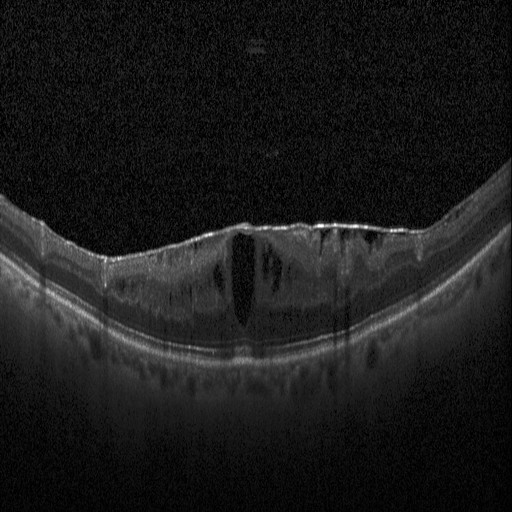

Acquired on a Heidelberg Spectralis · OCT line scan · spectral-domain optical coherence tomography. Assessment: diabetic macular edema (DME).